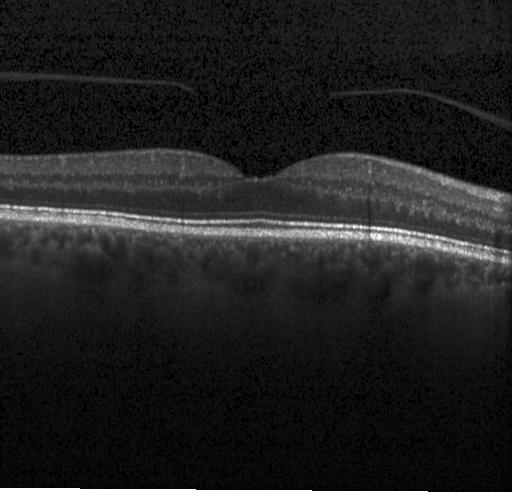 Retinal OCT cross-section.
Neither choroidal neovascularization, diabetic macular edema, nor drusen.